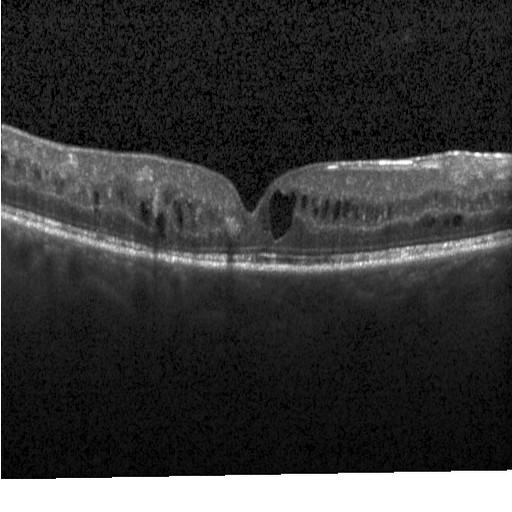

Assessment: DME.